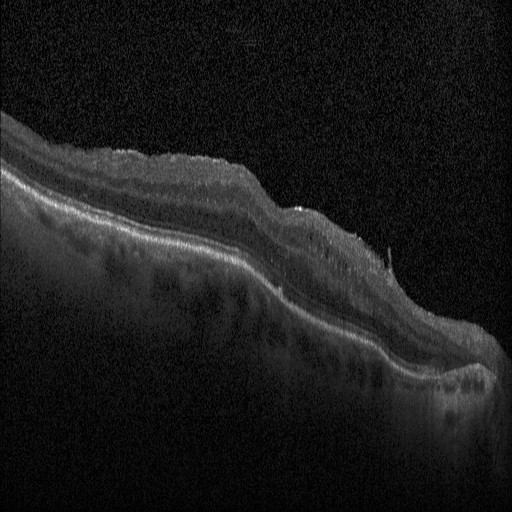 Assessment: DME.